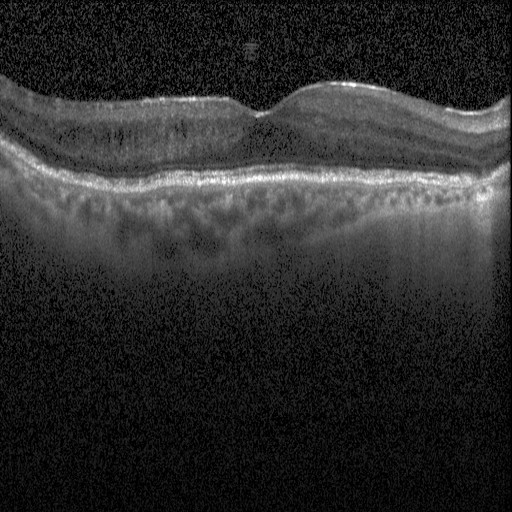
Retinal OCT cross-section. Impression: diabetic macular edema (DME).